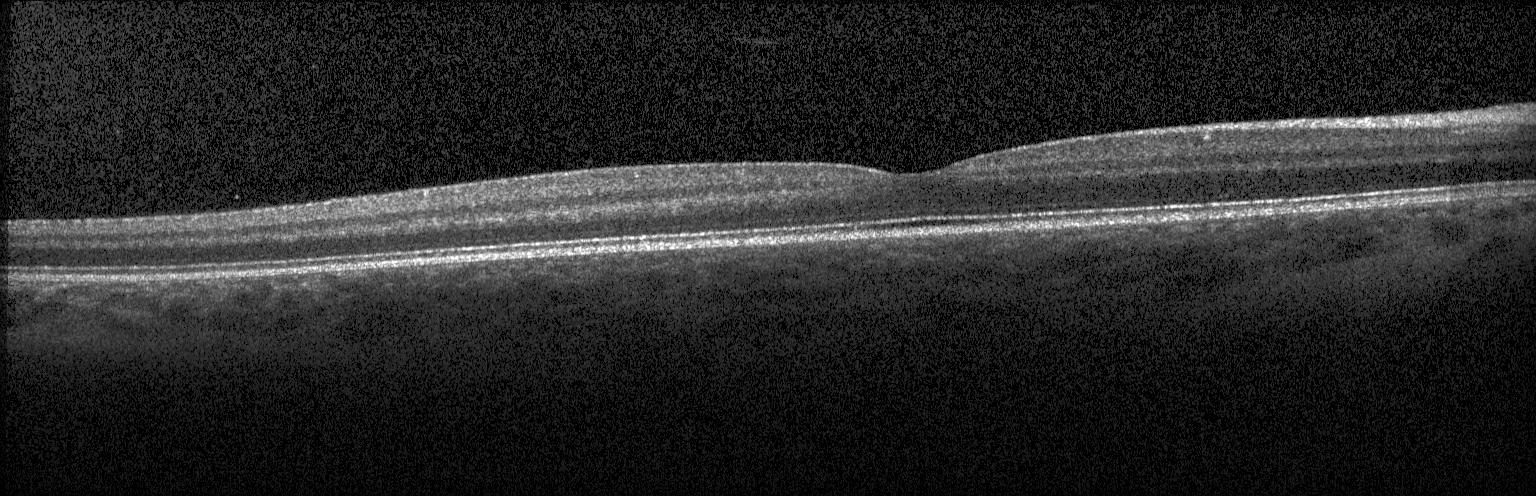

SD-OCT, acquired on a Heidelberg Spectralis, retinal OCT B-scan, fovea-centered
This B-scan demonstrates no CNV, no DME, and no drusen.